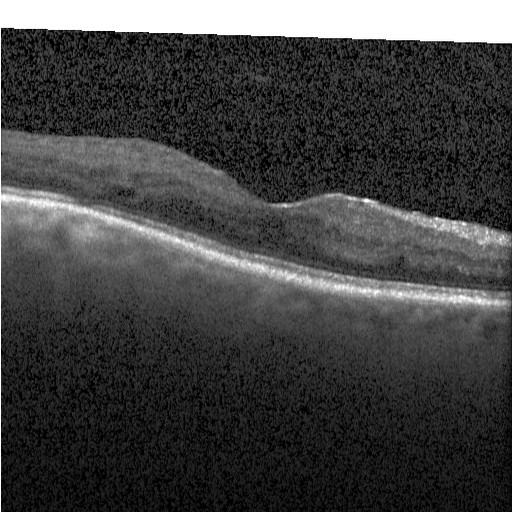

Macular OCT: diabetic macular edema.